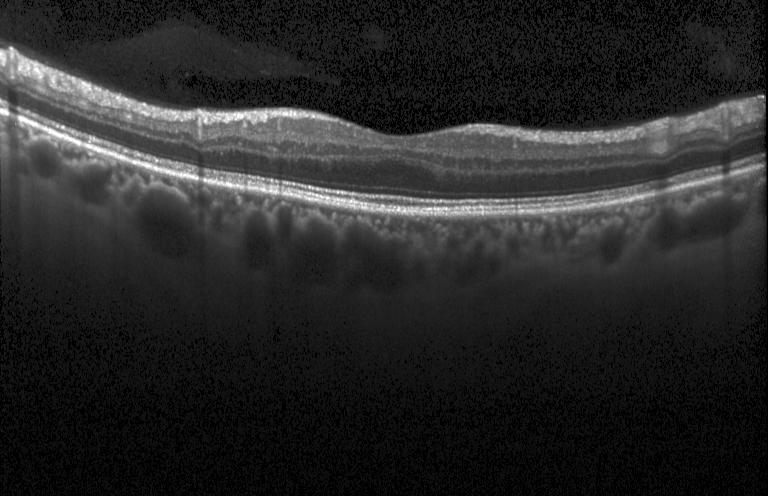 Neither choroidal neovascularization, diabetic macular edema, nor drusen.